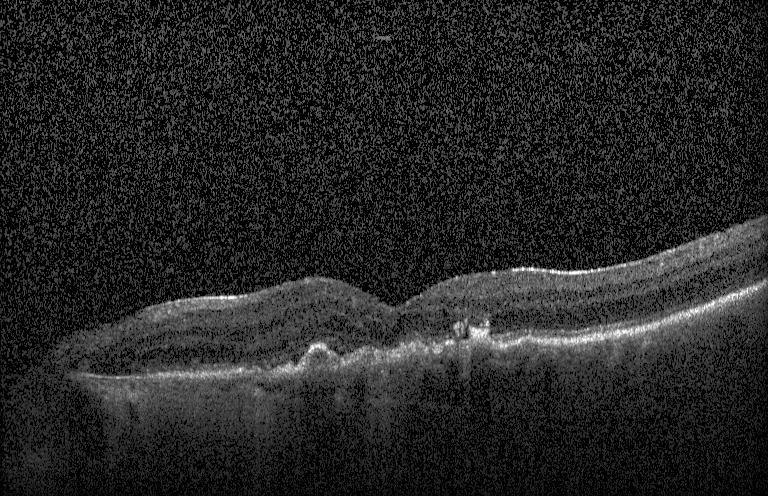

Retinal OCT cross-section showing CNV.